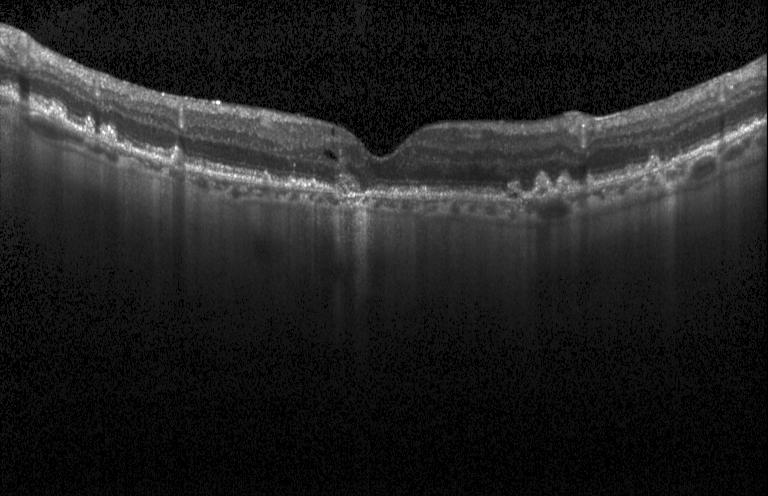

Dx: CNV.